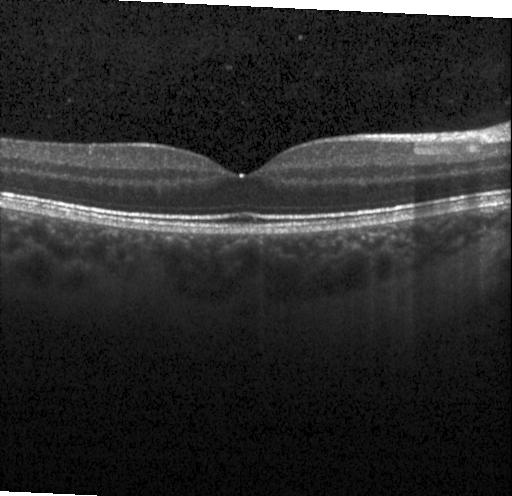
Retinal OCT cross-section. Spectral-domain OCT.
Finding: no evidence of CNV, DME, or drusen.